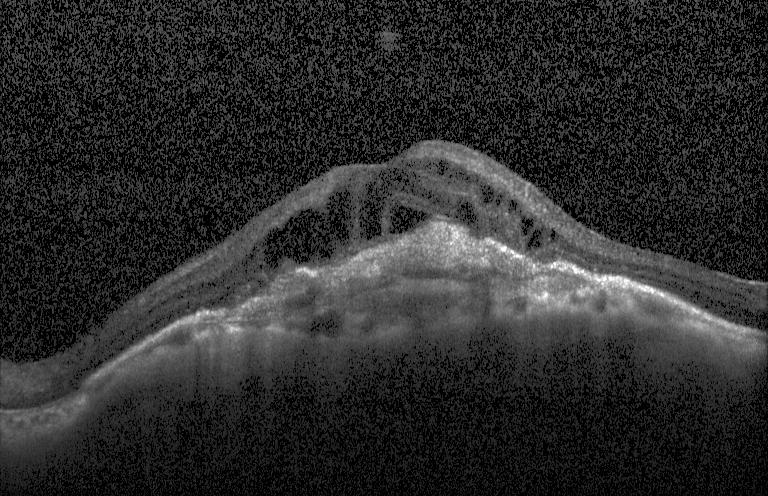

Macular OCT: a choroidal neovascular membrane.